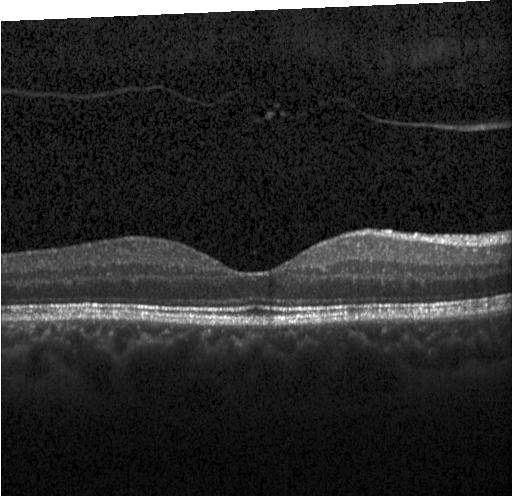

This B-scan demonstrates no choroidal neovascularization, diabetic macular edema, or drusen.